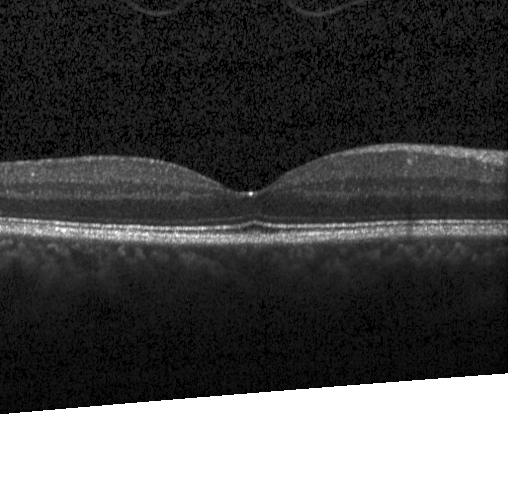

OCT line scan. Heidelberg Spectralis
OCT finding: neither choroidal neovascularization, diabetic macular edema, nor drusen.